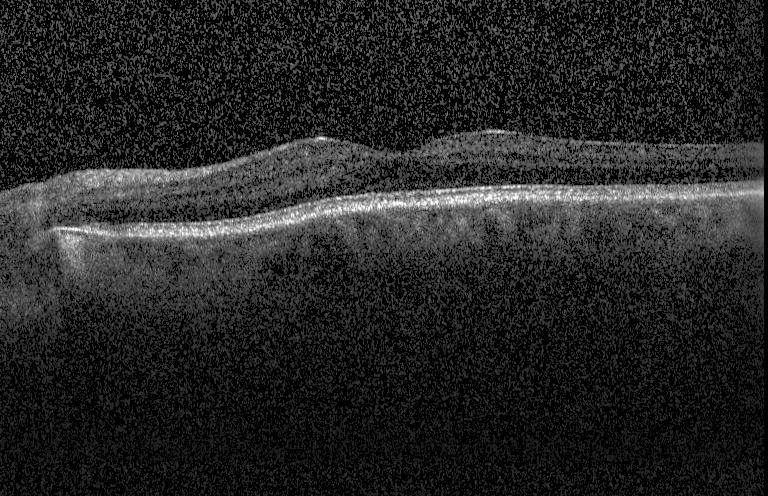
OCT B-scan · instrument: Heidelberg Spectralis · horizontal scan through the fovea.
Impression: no evidence of choroidal neovascularization, diabetic macular edema, or drusen.